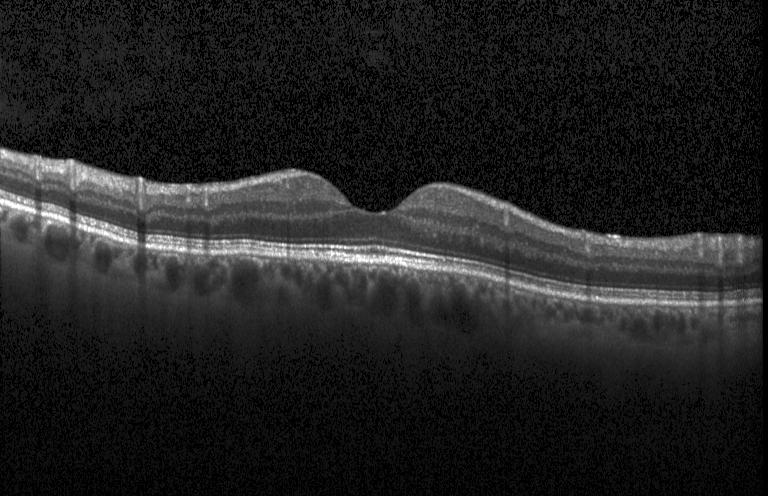

Heidelberg Spectralis OCT system · OCT B-scan.
Finding: neither CNV, DME, nor drusen.